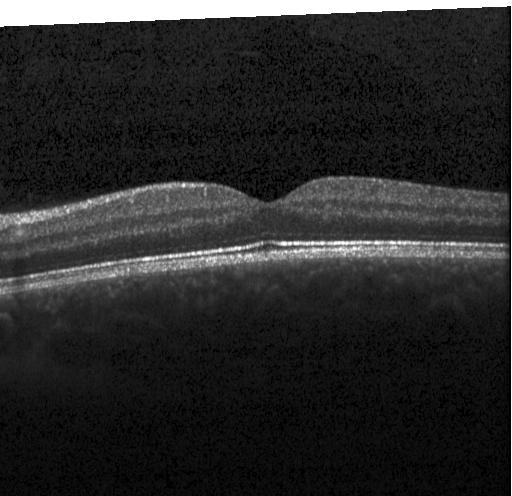
OCT finding: neither choroidal neovascularization, diabetic macular edema, nor drusen.